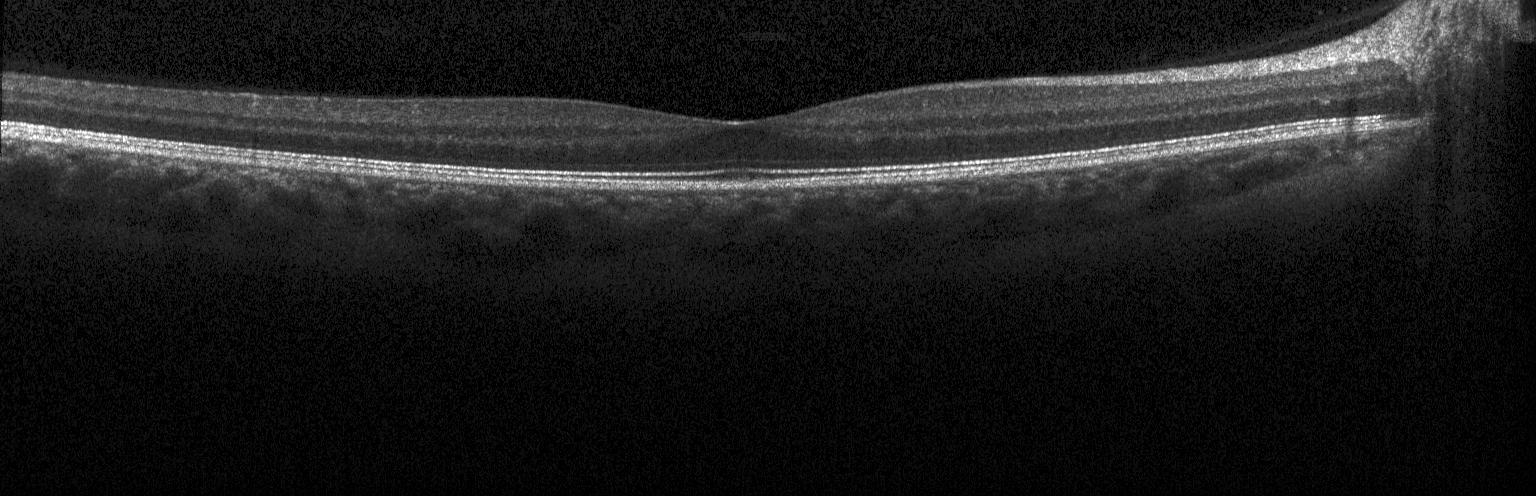
Diagnosis: neither CNV, DME, nor drusen.